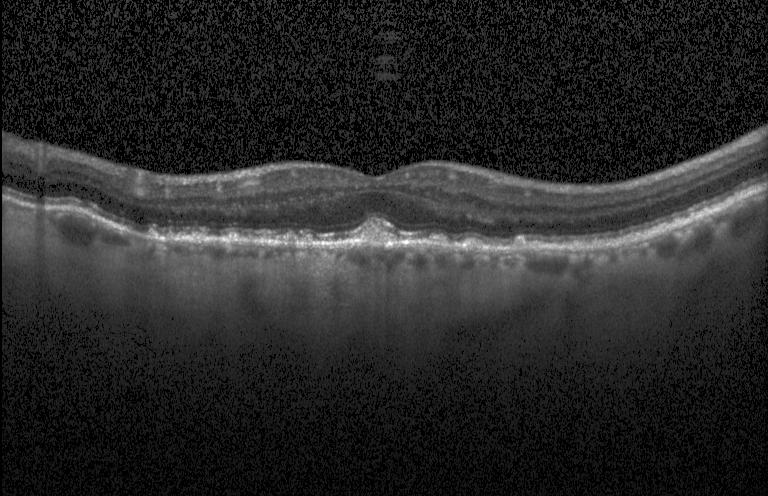 Spectral-domain OCT. OCT line scan
Dx: drusen.